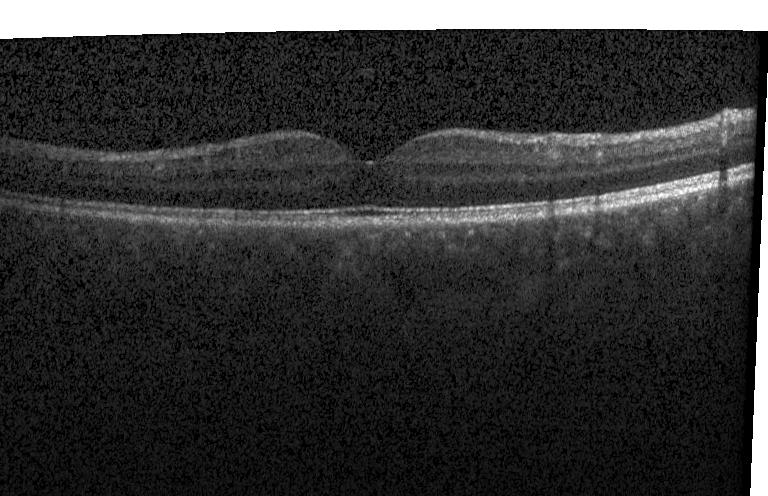
Diagnosis: no choroidal neovascularization, diabetic macular edema, or drusen.